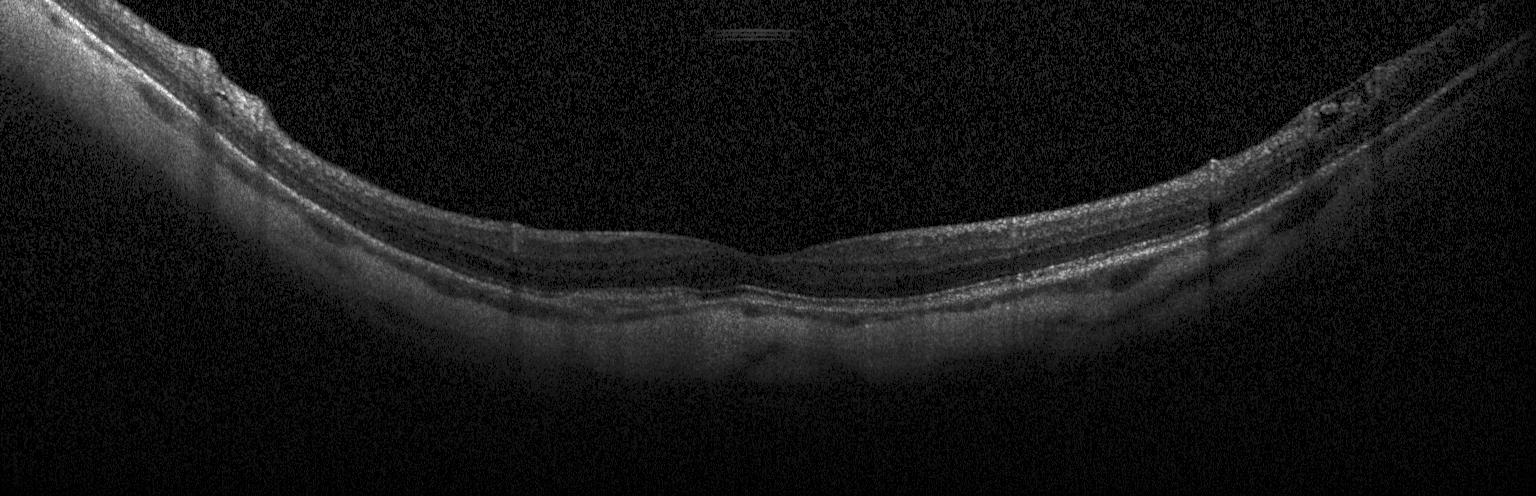
Retinal OCT B-scan. Choroidal neovascularization (CNV).